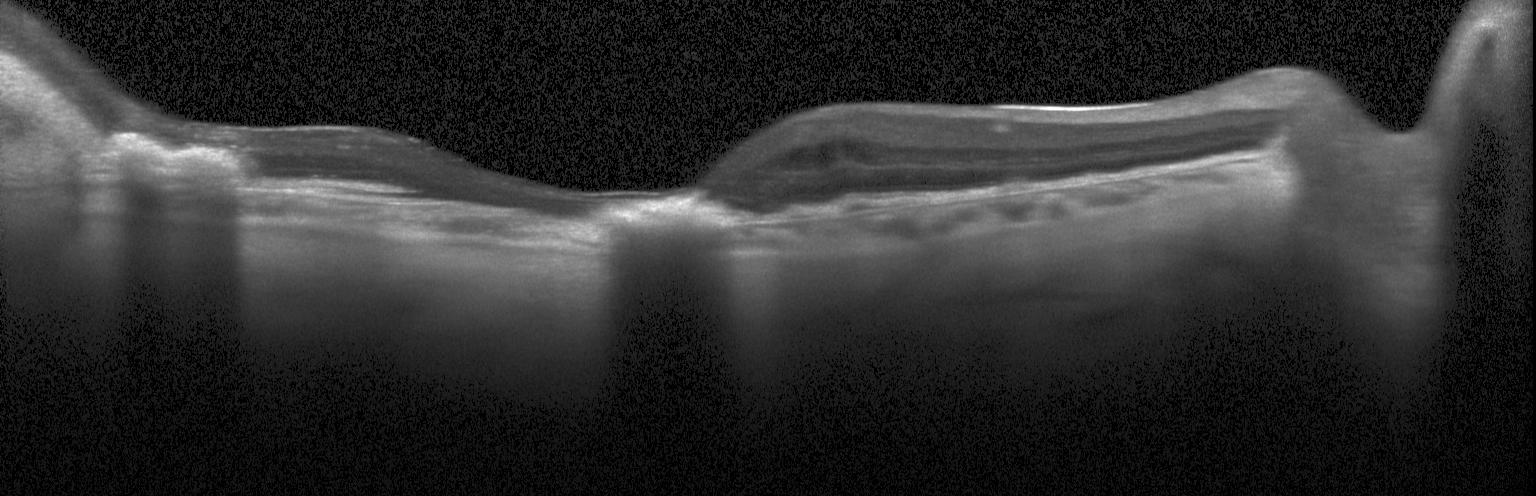
Retinal OCT B-scan, horizontal scan through the fovea.
Macular OCT: choroidal neovascularization.